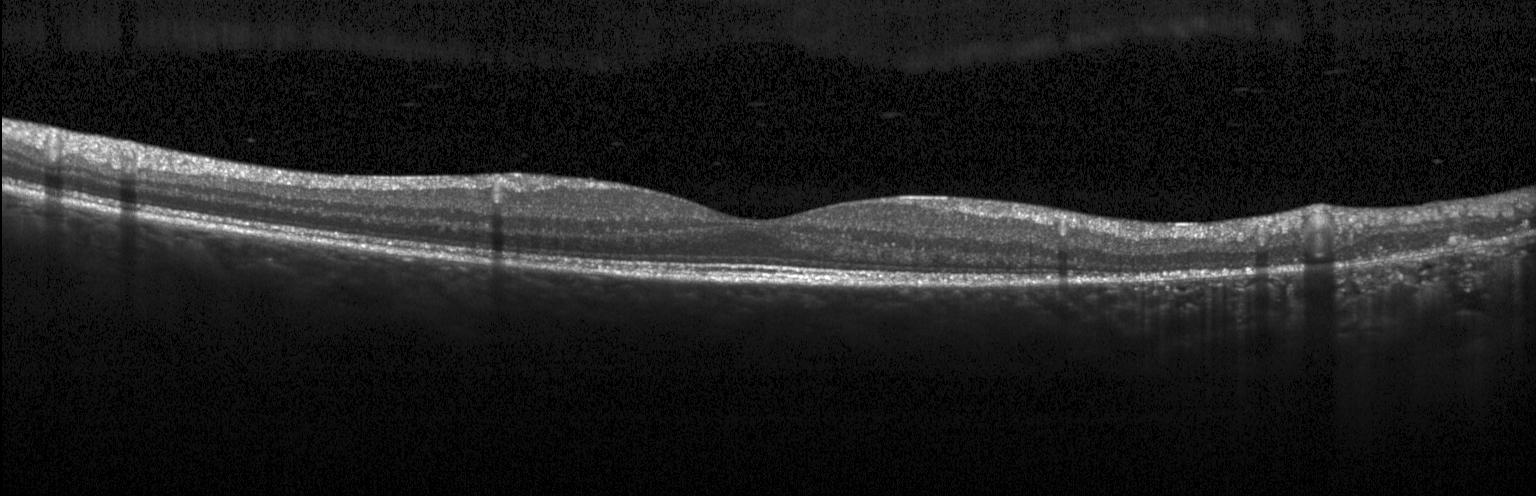

Spectral-domain OCT · retinal OCT B-scan · Heidelberg Spectralis OCT system
OCT finding: neither CNV, DME, nor drusen.